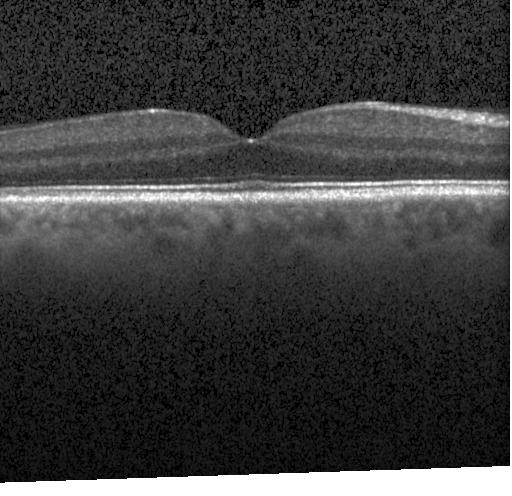
OCT line scan · macular scan · Heidelberg Spectralis OCT system — Impression: no choroidal neovascularization, no diabetic macular edema, and no drusen.